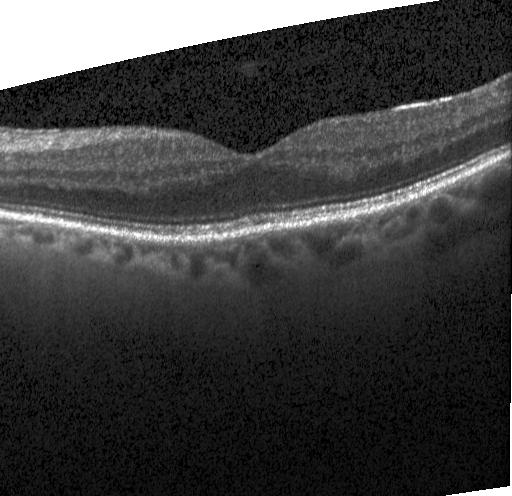
SD-OCT; optical coherence tomography B-scan; centered on the fovea — Macular OCT: neither choroidal neovascularization, diabetic macular edema, nor drusen.